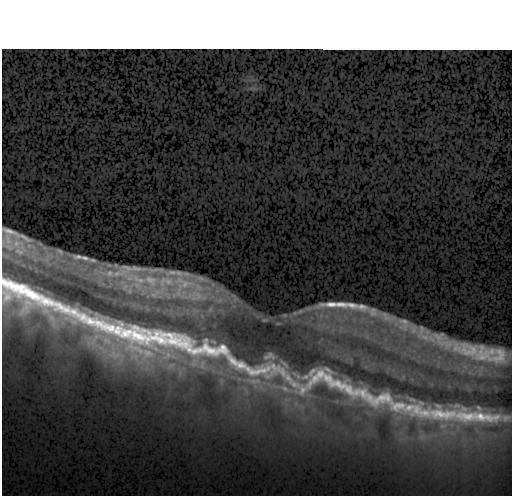 Retinal OCT B-scan
Choroidal neovascularization.